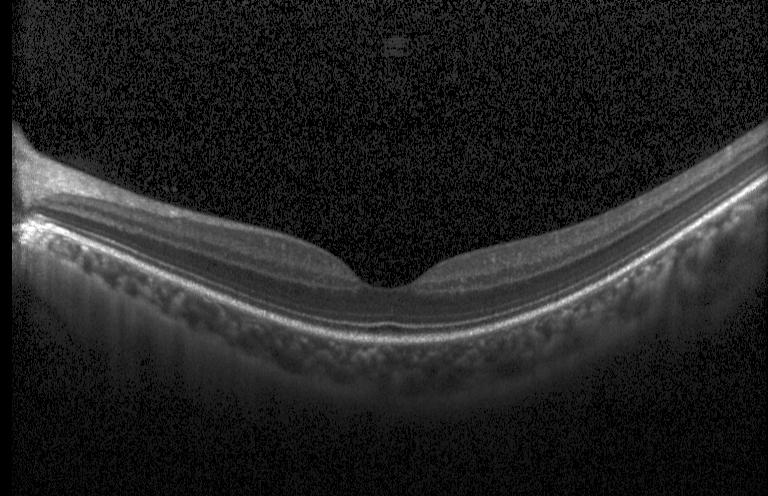

Impression: no choroidal neovascularization, no diabetic macular edema, and no drusen.